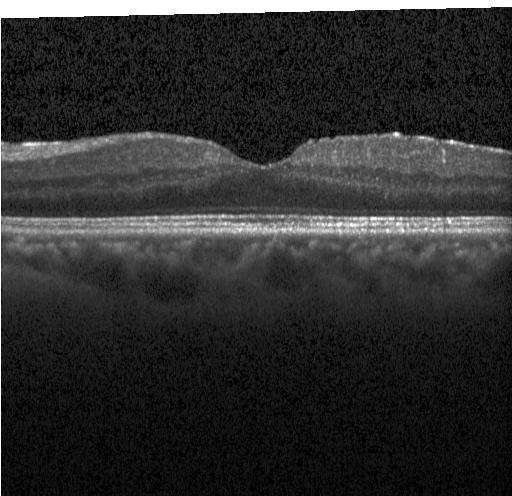 Horizontal scan through the fovea; Heidelberg Spectralis OCT system; OCT line scan; spectral-domain OCT — Impression: no evidence of choroidal neovascularization, diabetic macular edema, or drusen.